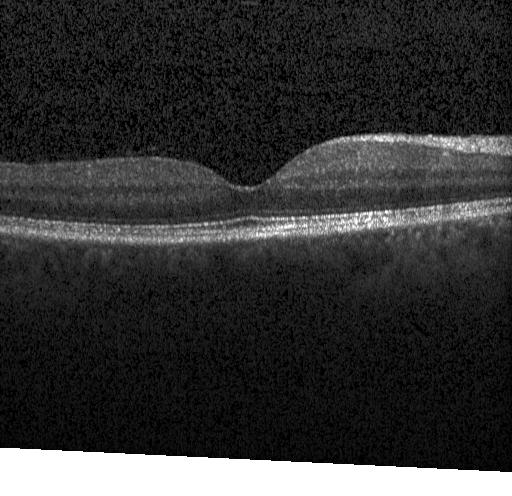 Spectral-domain OCT B-scan: no CNV, DME, or drusen.